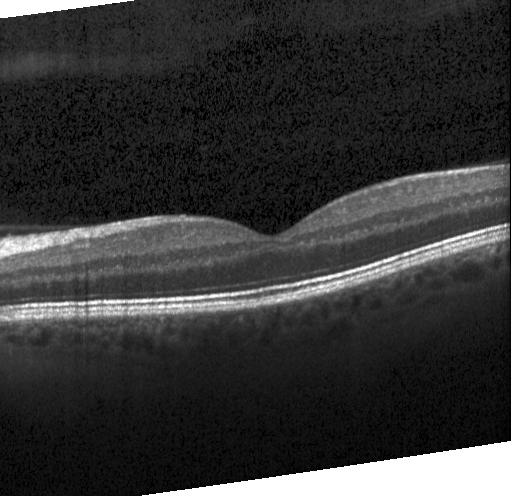 Assessment: no evidence of CNV, DME, or drusen.